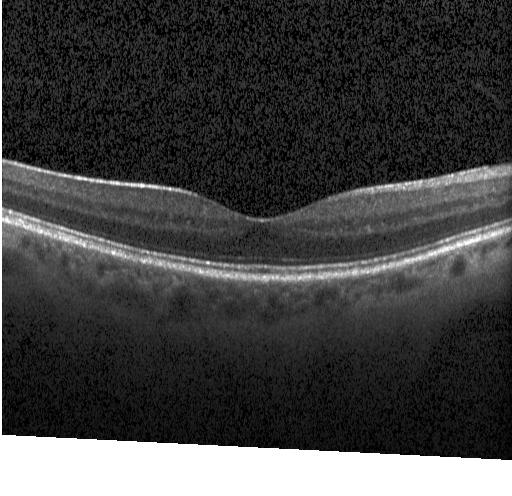

Finding: neither choroidal neovascularization, diabetic macular edema, nor drusen.